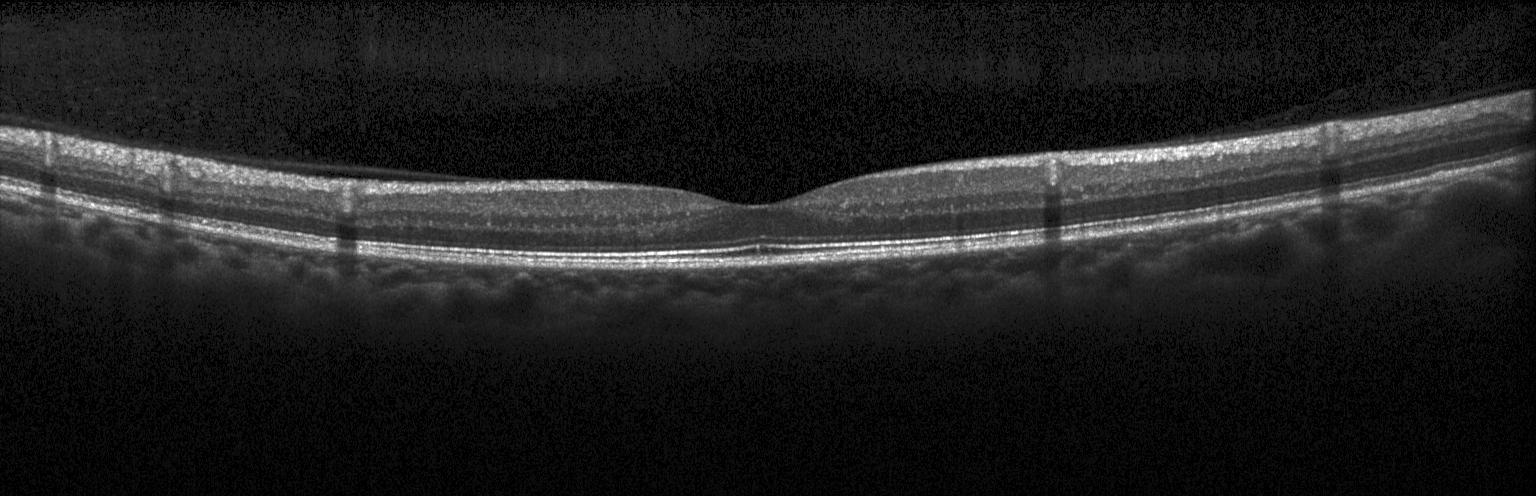 Optical coherence tomography B-scan, SD-OCT.
Macular OCT: no evidence of CNV, DME, or drusen.